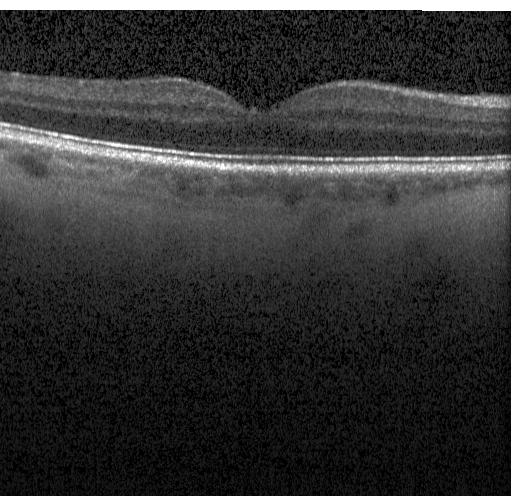
Optical coherence tomography B-scan. Centered on the fovea. Impression: no evidence of CNV, DME, or drusen.